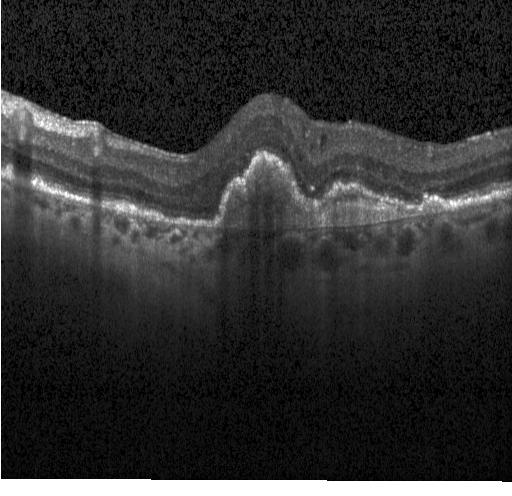 OCT finding: CNV.